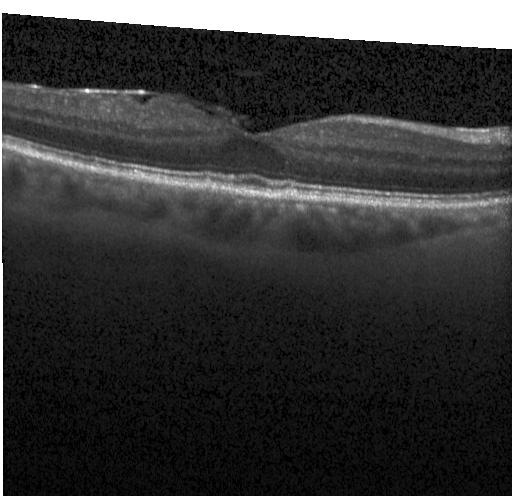

Horizontal scan through the fovea. Acquired on a Heidelberg Spectralis. Retinal OCT B-scan — This B-scan demonstrates drusen.